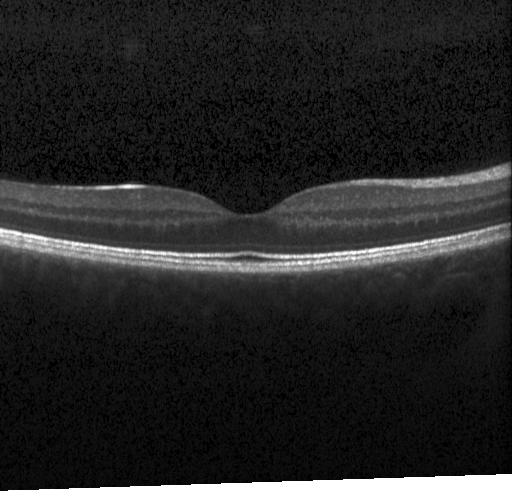
Spectral-domain optical coherence tomography · acquired on a Heidelberg Spectralis · OCT line scan · centered on the fovea.
Neither choroidal neovascularization, diabetic macular edema, nor drusen.